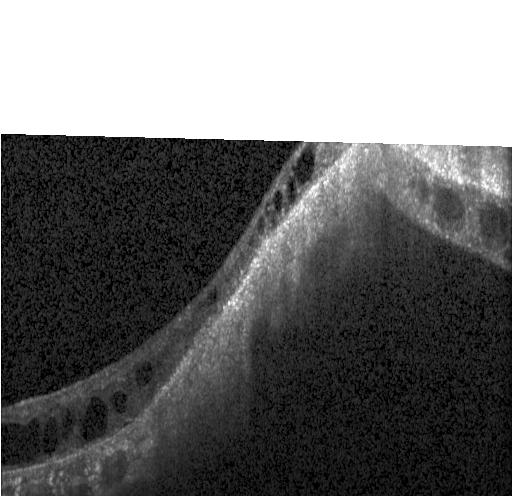 OCT scan showing diabetic macular edema (DME).